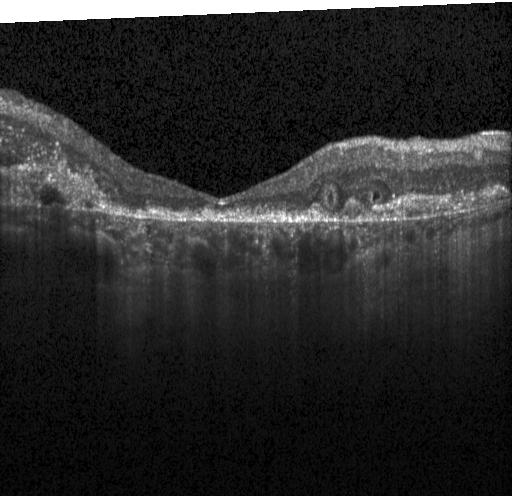 Optical coherence tomography scan.
Macular OCT: a choroidal neovascular membrane.